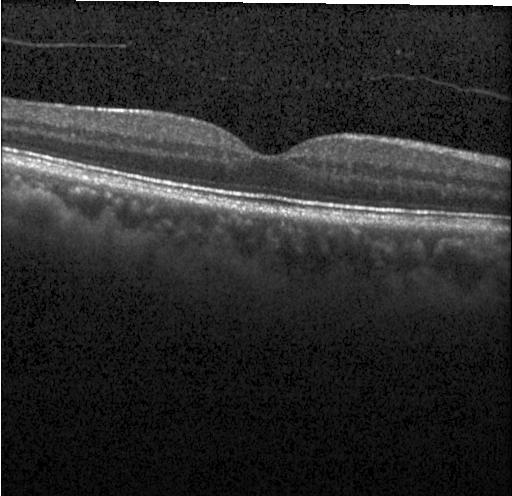
Spectral-domain OCT B-scan: no choroidal neovascularization, diabetic macular edema, or drusen.